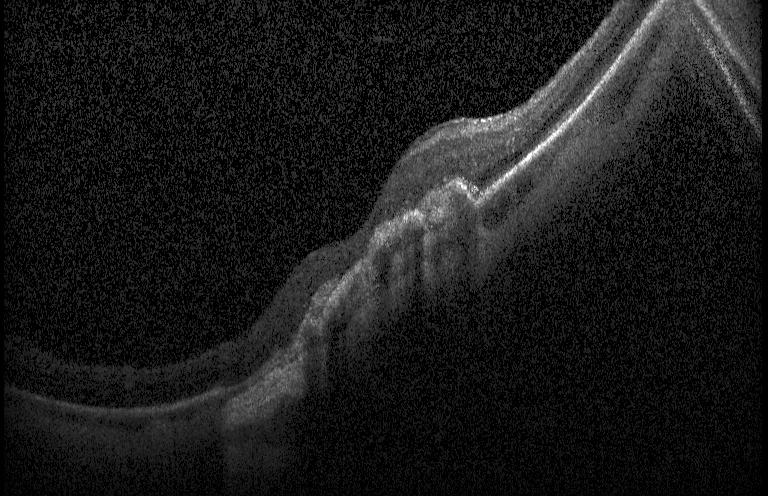
Retinal OCT B-scan · through the macula · SD-OCT · instrument: Heidelberg Spectralis
Dx: choroidal neovascularization.